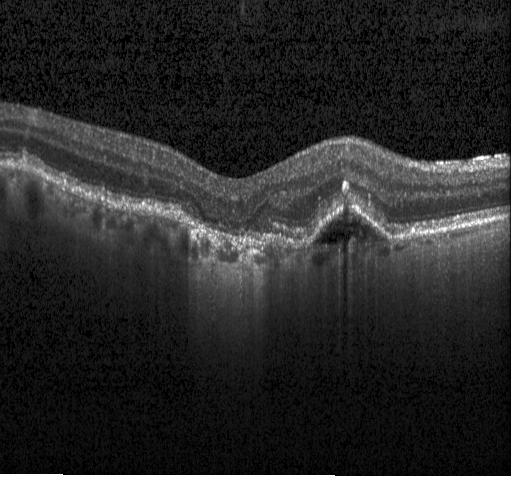
Optical coherence tomography B-scan. Assessment: CNV.